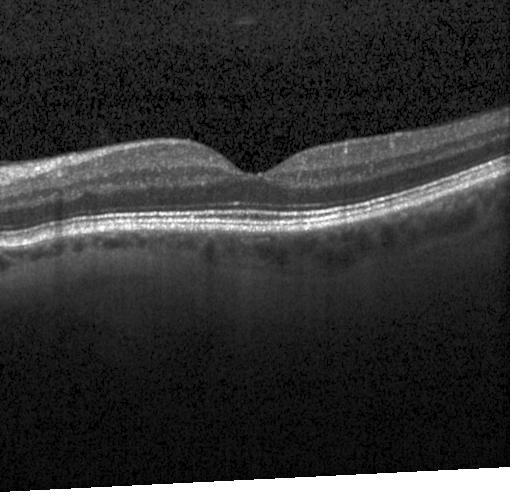 Heidelberg Spectralis OCT system, OCT line scan.
Assessment: no evidence of CNV, DME, or drusen.